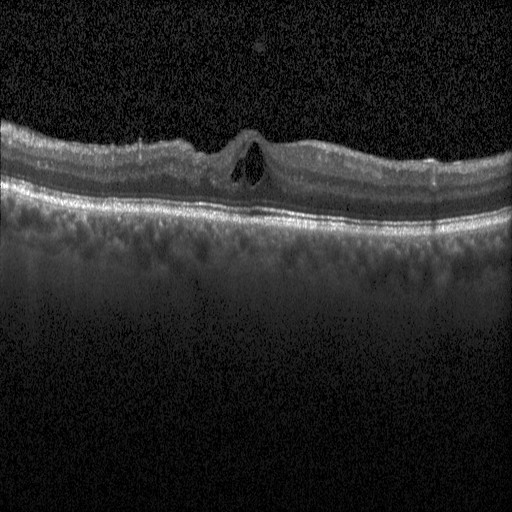

Finding: diabetic macular edema (DME).